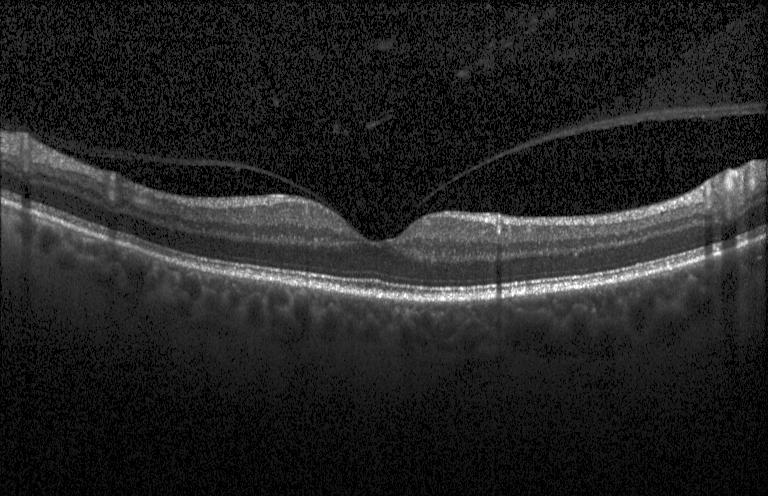

Optical coherence tomography scan · Heidelberg Spectralis — No choroidal neovascularization, no diabetic macular edema, and no drusen.